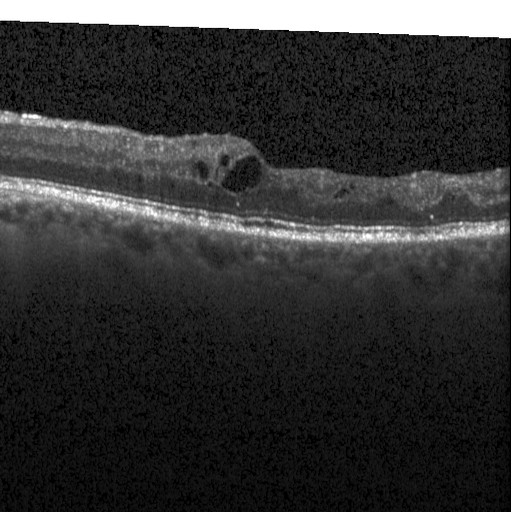

Retinal OCT B-scan; macular scan; acquired on a Heidelberg Spectralis; SD-OCT — Diagnosis: diabetic macular edema (DME).